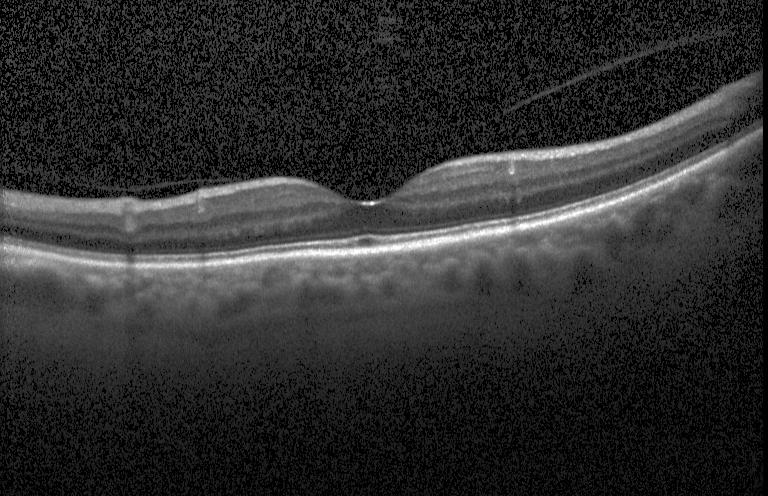

Retinal OCT cross-section. SD-OCT. The scan shows no evidence of choroidal neovascularization, diabetic macular edema, or drusen.